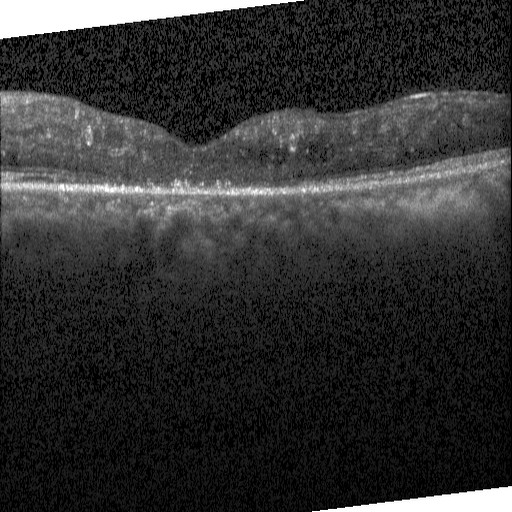 OCT finding: diabetic macular edema.